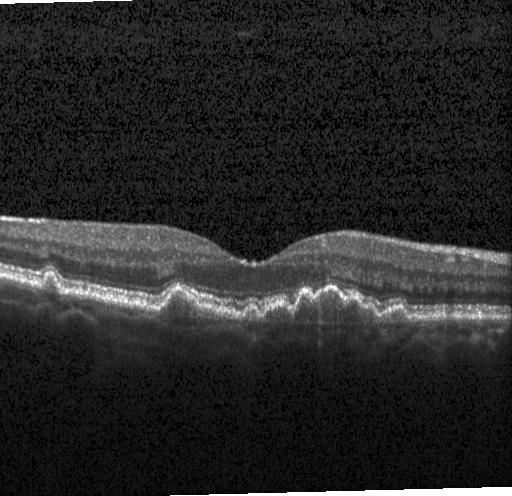
SD-OCT, optical coherence tomography scan. Finding: drusen.